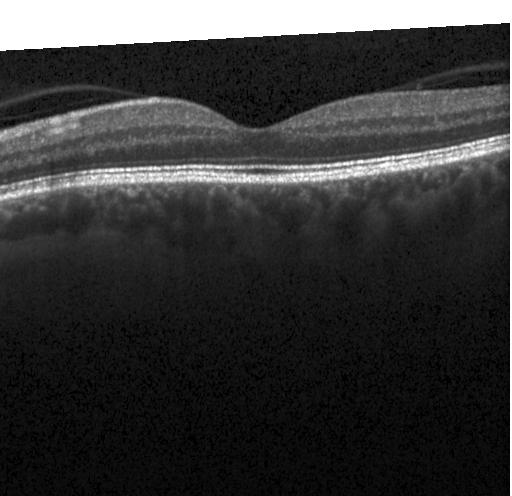 OCT finding: no choroidal neovascularization, diabetic macular edema, or drusen.